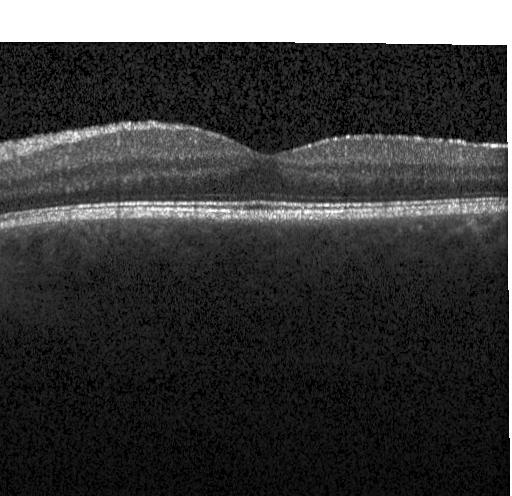 Retinal OCT B-scan — Assessment: no evidence of choroidal neovascularization, diabetic macular edema, or drusen.